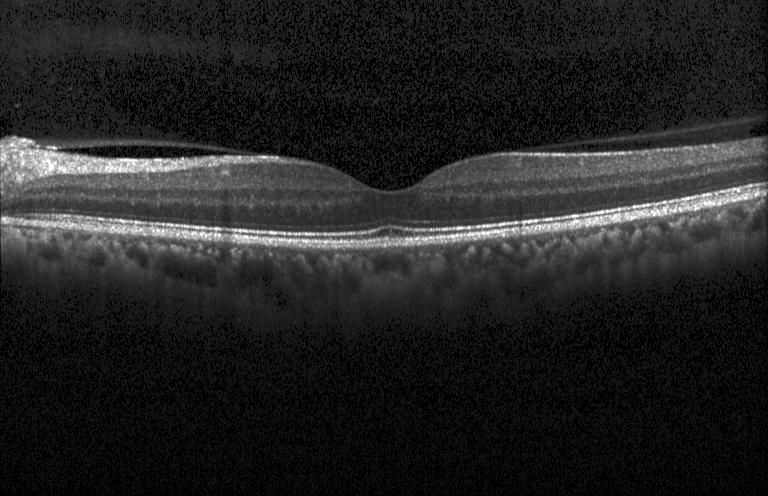
Optical coherence tomography scan — Dx: no evidence of CNV, DME, or drusen.